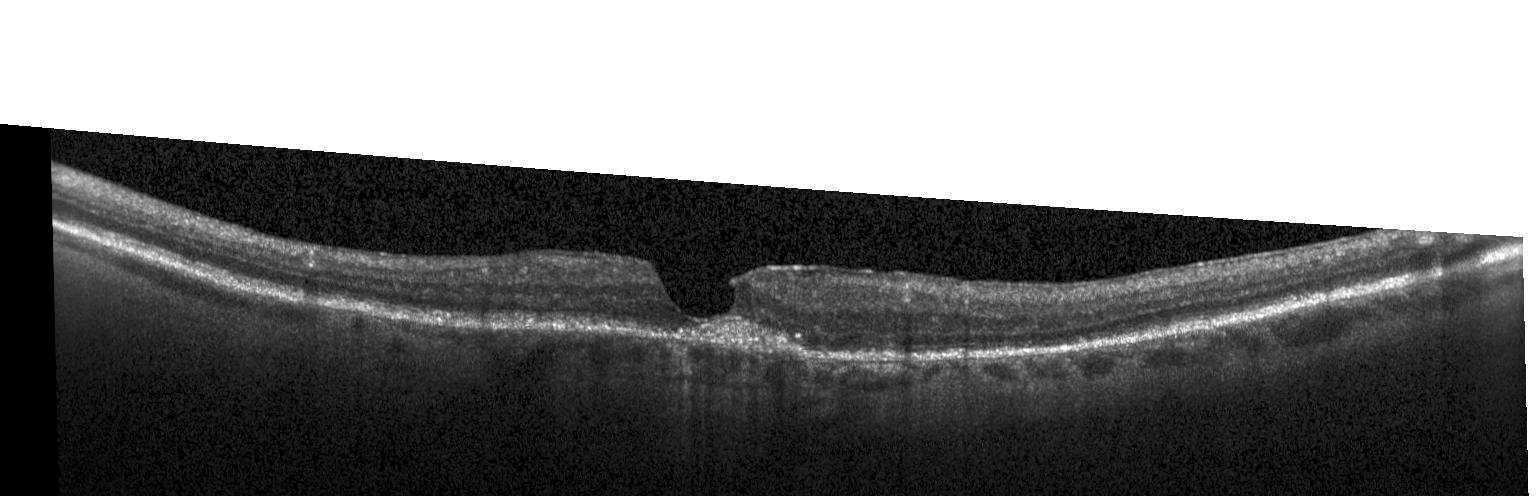

Impression: CNV.